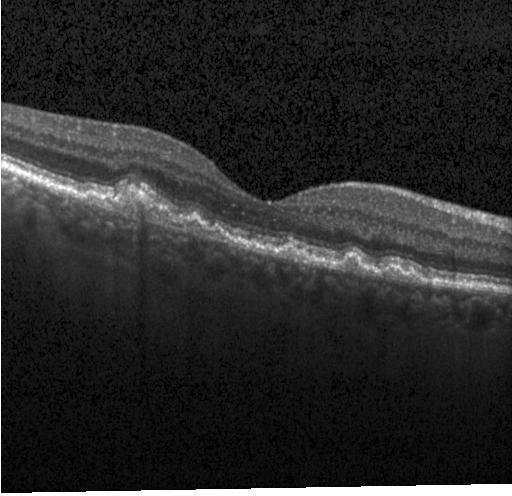 Macular OCT demonstrating choroidal neovascularization.